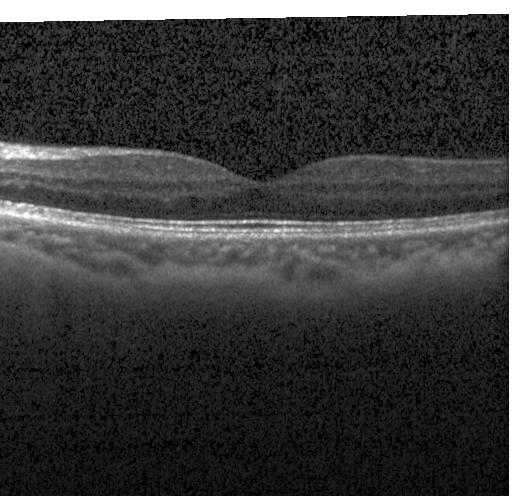 Impression: no evidence of choroidal neovascularization, diabetic macular edema, or drusen.